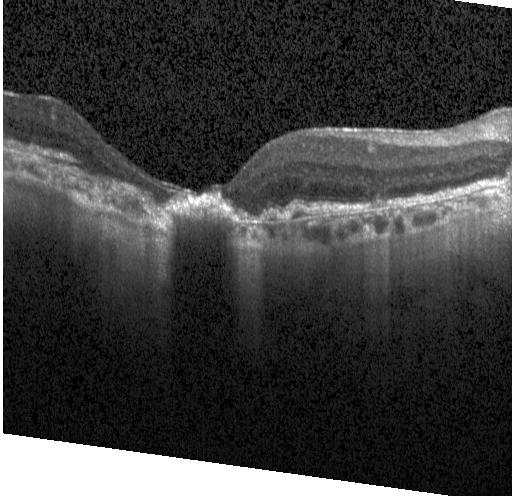

Macular OCT: choroidal neovascularization (CNV).